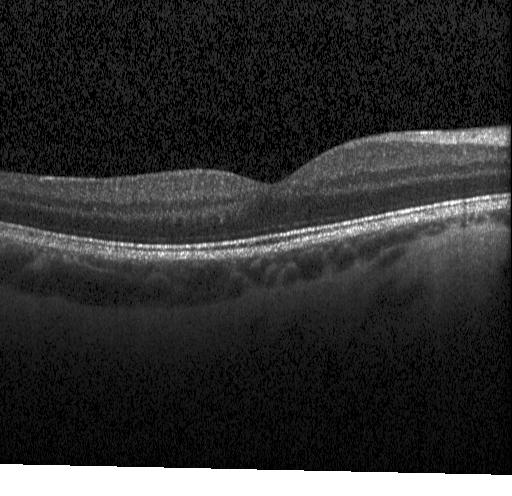
Heidelberg Spectralis; retinal OCT B-scan; macular scan
Diagnosis: neither CNV, DME, nor drusen.